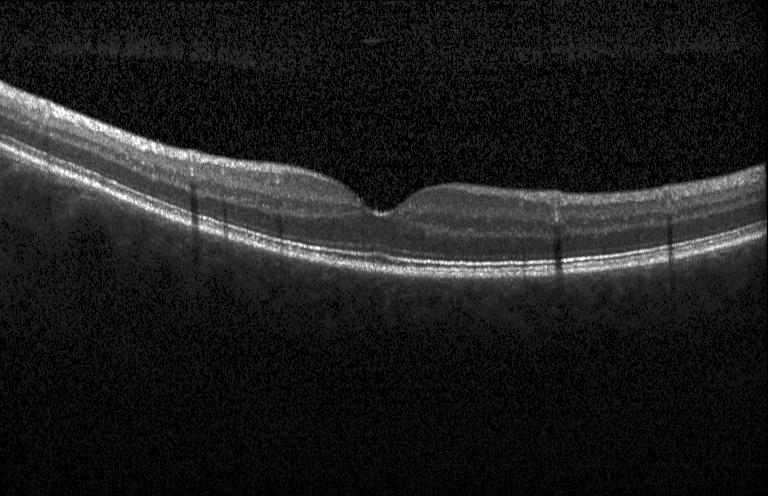
Retinal OCT B-scan. Heidelberg Spectralis. OCT finding: no CNV, DME, or drusen.